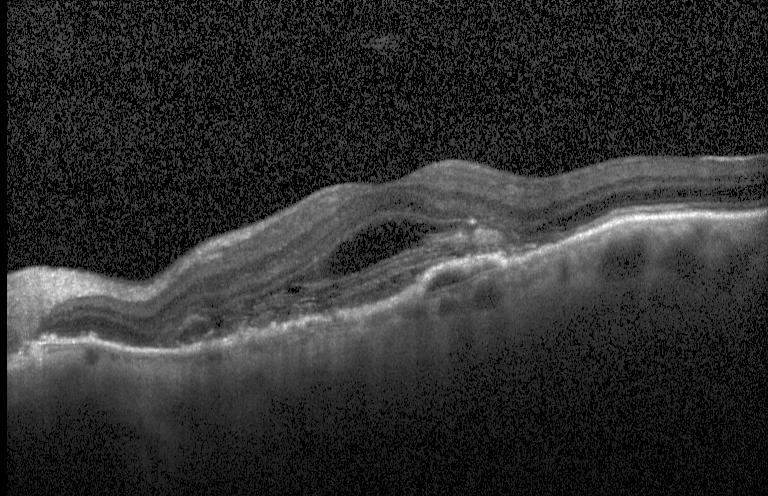 OCT finding: a choroidal neovascular membrane.